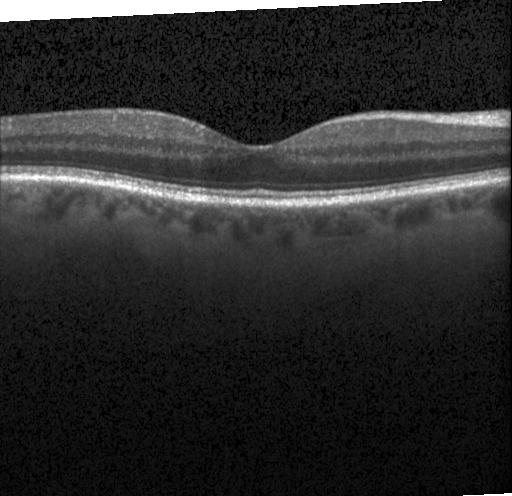
Optical coherence tomography B-scan. Heidelberg Spectralis. Through the macula. SD-OCT.
Impression: neither choroidal neovascularization, diabetic macular edema, nor drusen.